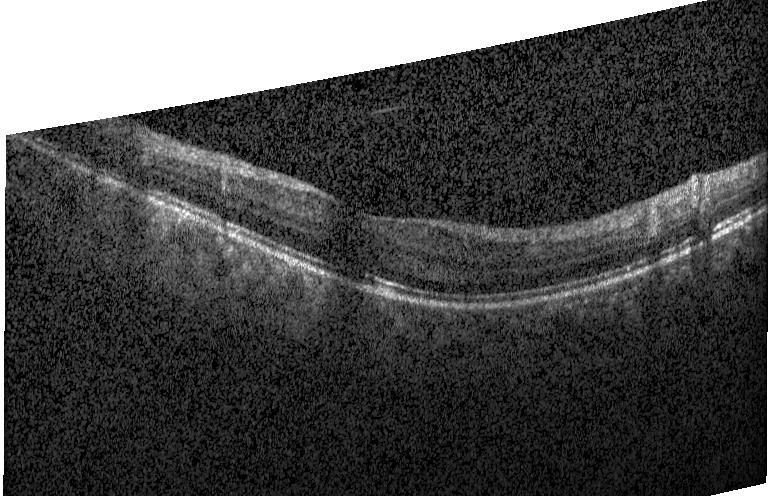

Assessment: no evidence of choroidal neovascularization, diabetic macular edema, or drusen.